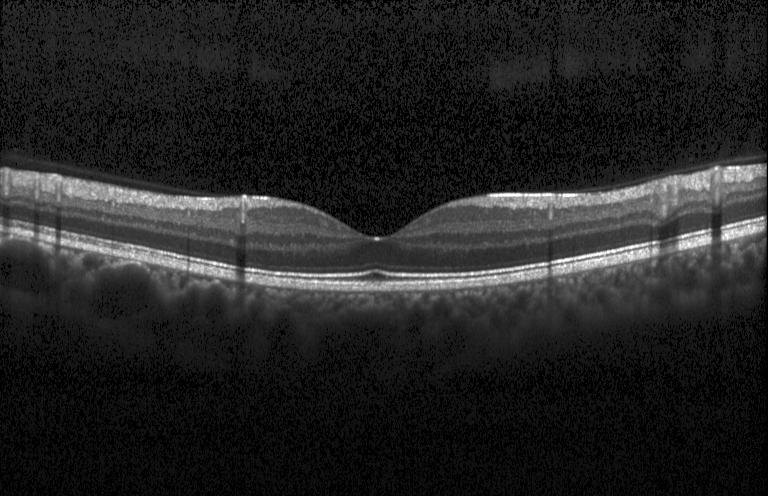
Acquired on a Heidelberg Spectralis · OCT B-scan. No choroidal neovascularization, no diabetic macular edema, and no drusen.